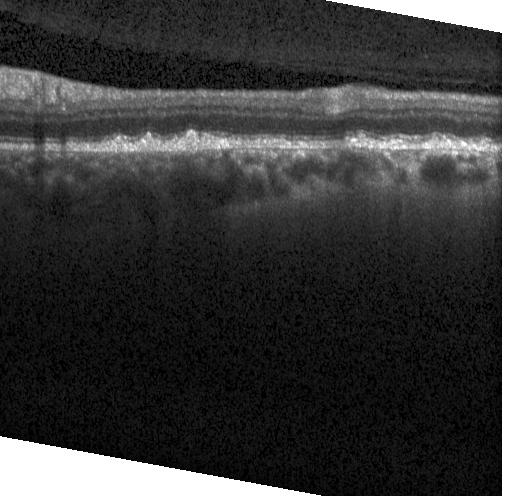

Retinal OCT B-scan · SD-OCT — Diagnosis: drusen.